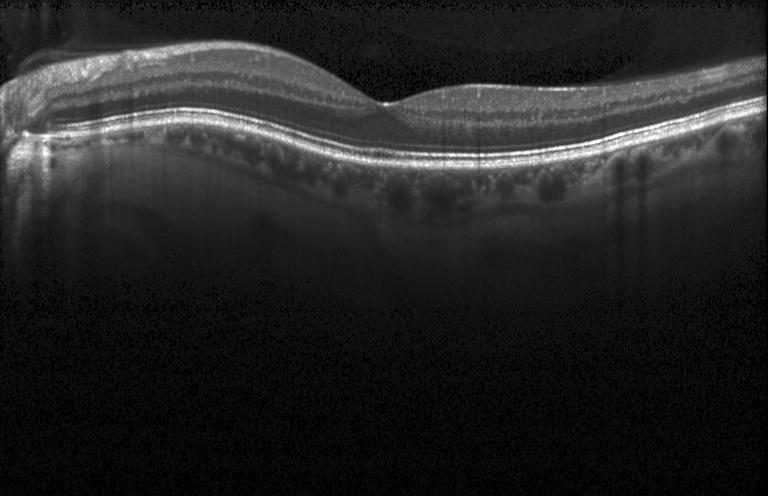
Finding: no choroidal neovascularization, no diabetic macular edema, and no drusen.